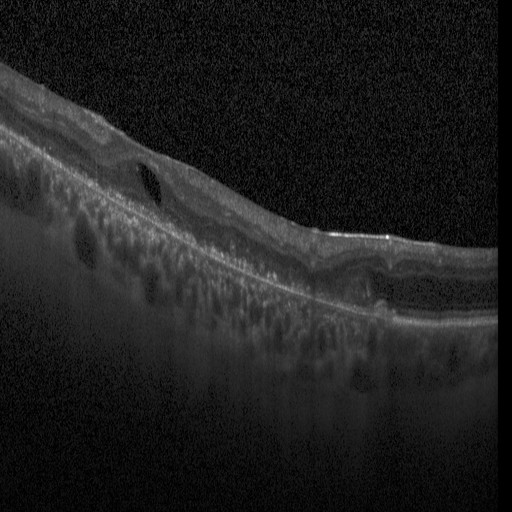

Optical coherence tomography B-scan. Assessment: diabetic macular edema (DME).